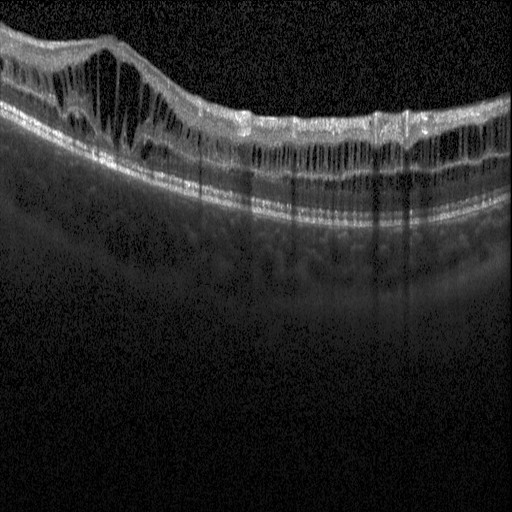
Retinal OCT B-scan, horizontal scan through the fovea, spectral-domain OCT. The scan shows DME.